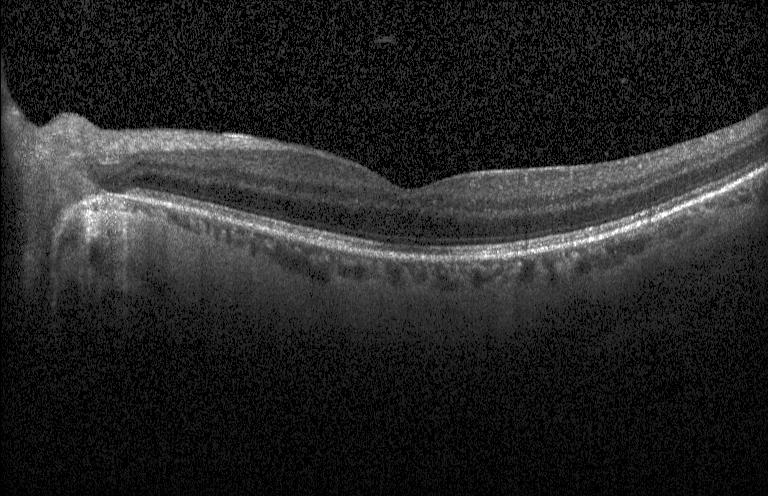

The scan shows no evidence of CNV, DME, or drusen.